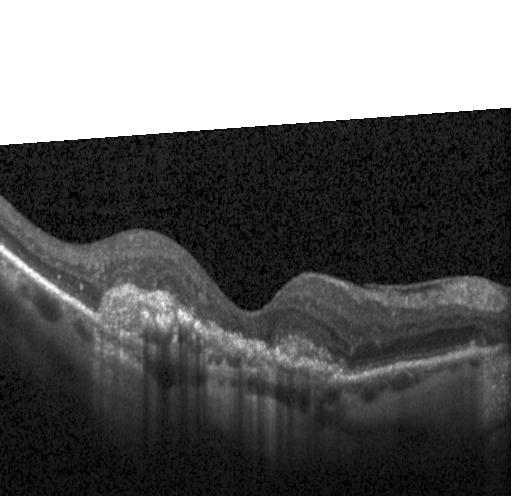
Optical coherence tomography B-scan.
Macular OCT: a choroidal neovascular membrane.